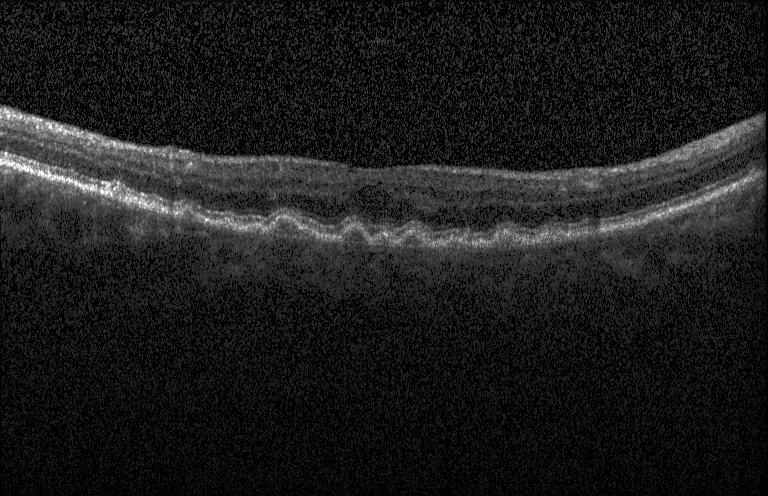

Finding: multiple drusen.